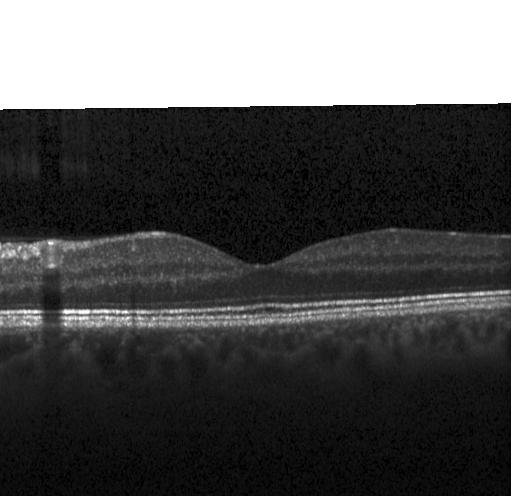
Instrument: Heidelberg Spectralis; retinal OCT B-scan; SD-OCT. Macular OCT: no CNV, DME, or drusen.